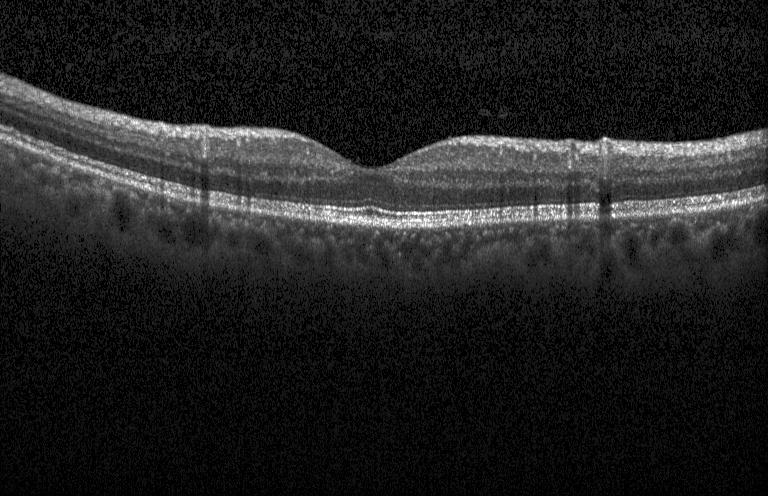

OCT line scan. Instrument: Heidelberg Spectralis. Spectral-domain OCT — This B-scan demonstrates no evidence of choroidal neovascularization, diabetic macular edema, or drusen.